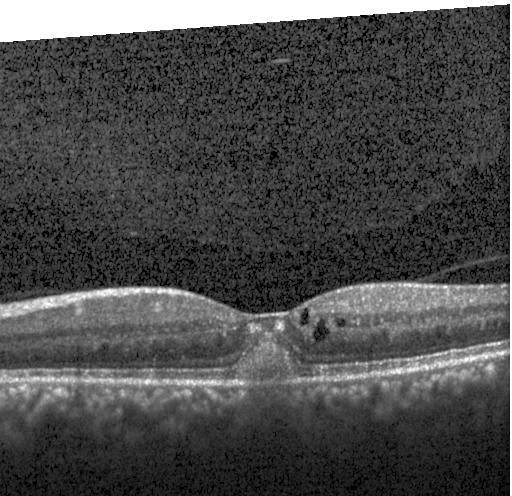

Diagnosis: a choroidal neovascular membrane.